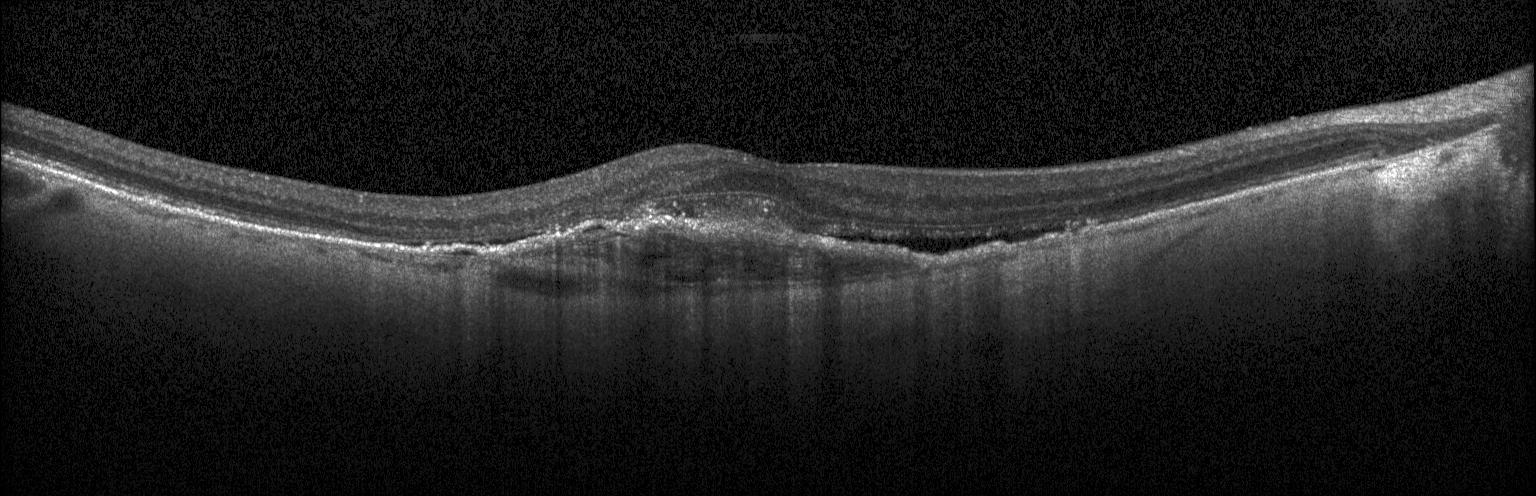
The scan shows a choroidal neovascular membrane.